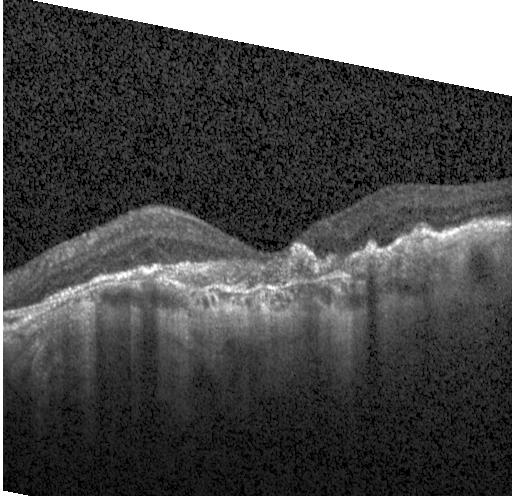 Acquired on a Heidelberg Spectralis, optical coherence tomography scan, through the macula. Assessment: CNV.